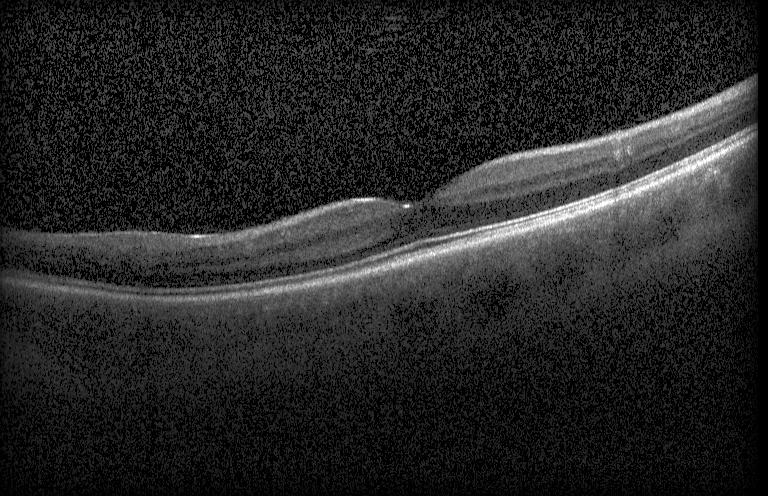
Centered on the fovea. Optical coherence tomography B-scan. Acquired on a Heidelberg Spectralis. SD-OCT
OCT finding: no choroidal neovascularization, no diabetic macular edema, and no drusen.